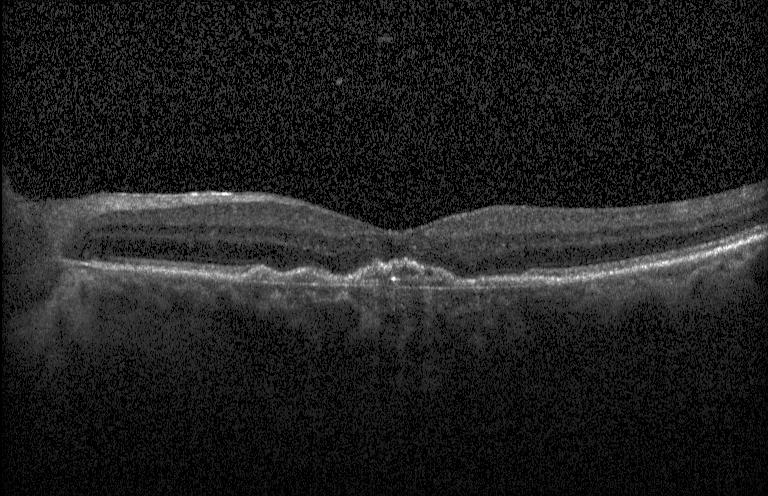

Retinal OCT cross-section
Assessment: a choroidal neovascular membrane.